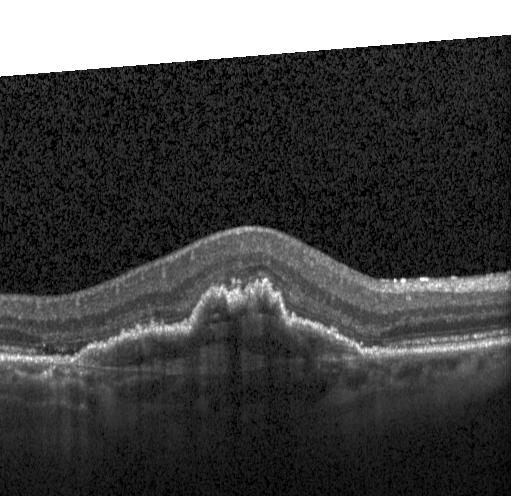 Optical coherence tomography scan, Heidelberg Spectralis, spectral-domain OCT.
Assessment: choroidal neovascularization.